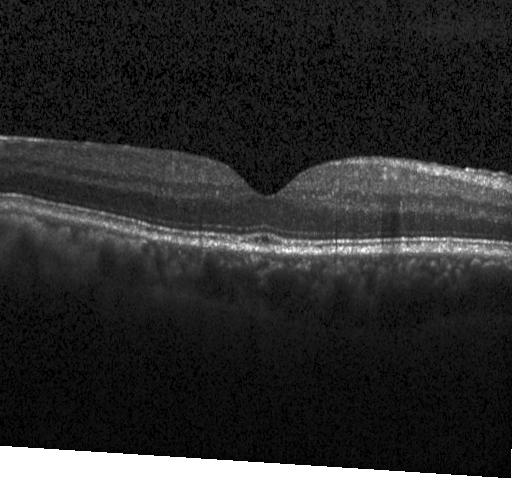

Optical coherence tomography B-scan; spectral-domain optical coherence tomography.
Assessment: no evidence of choroidal neovascularization, diabetic macular edema, or drusen.